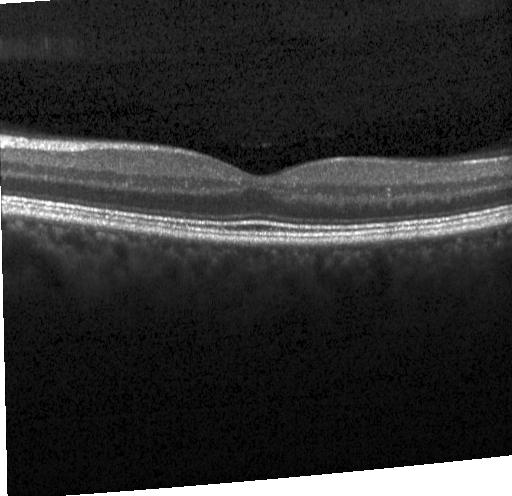

OCT line scan. Instrument: Heidelberg Spectralis. Centered on the fovea. SD-OCT
Diagnosis: no choroidal neovascularization, diabetic macular edema, or drusen.